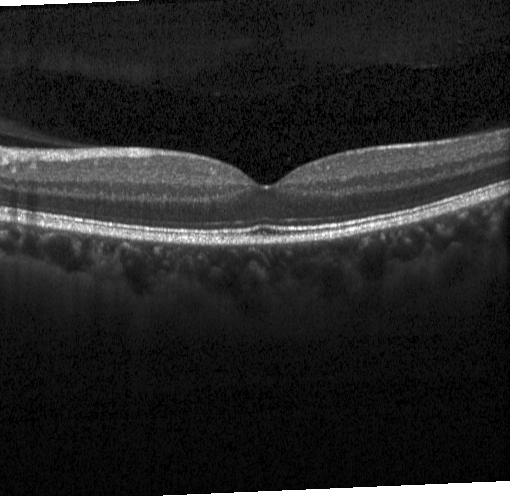
Through the macula. SD-OCT. Retinal OCT cross-section. Acquired on a Heidelberg Spectralis.
Impression: no evidence of CNV, DME, or drusen.